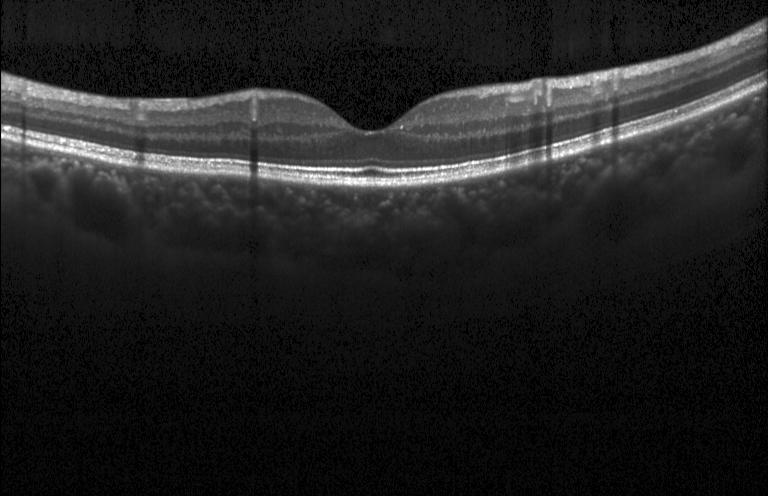

Acquired on a Heidelberg Spectralis; spectral-domain optical coherence tomography; fovea-centered; retinal OCT cross-section.
No CNV, DME, or drusen.